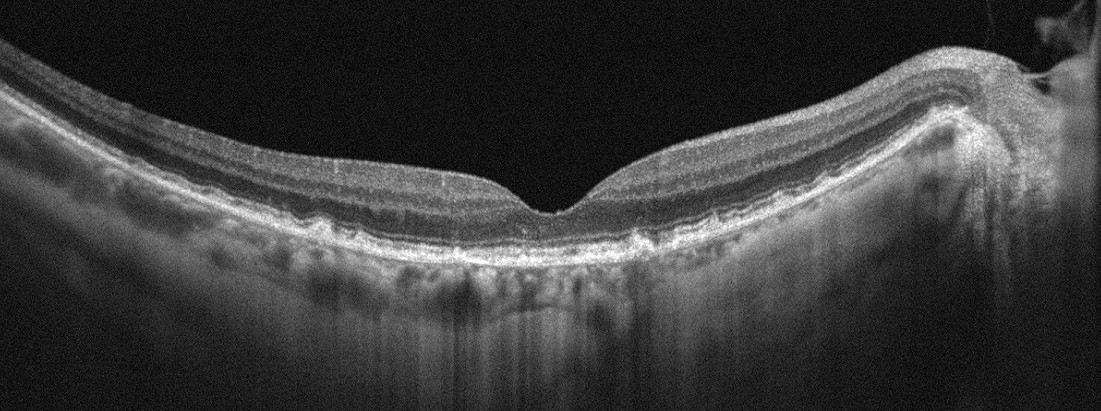
Instrument: Optovue Avanti RTVue XR · OCT line scan. Age-related macular degeneration.